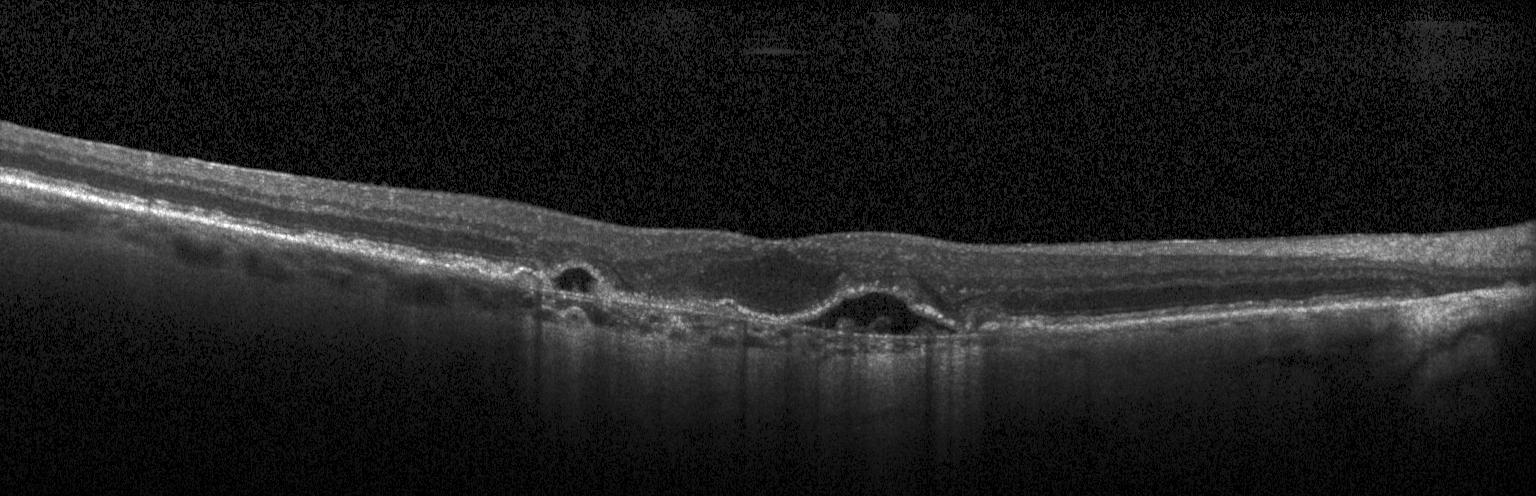

OCT line scan. Macular OCT: a choroidal neovascular membrane.